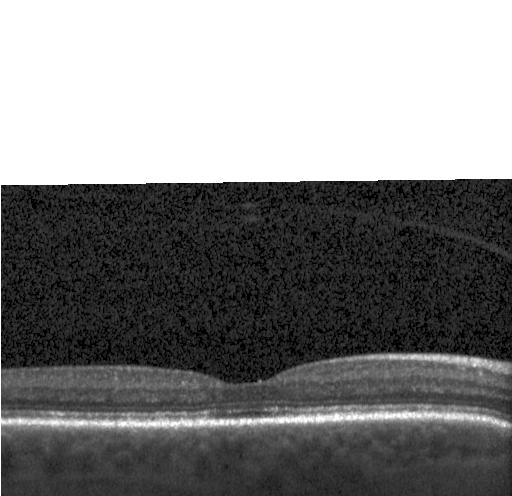 No CNV, DME, or drusen.